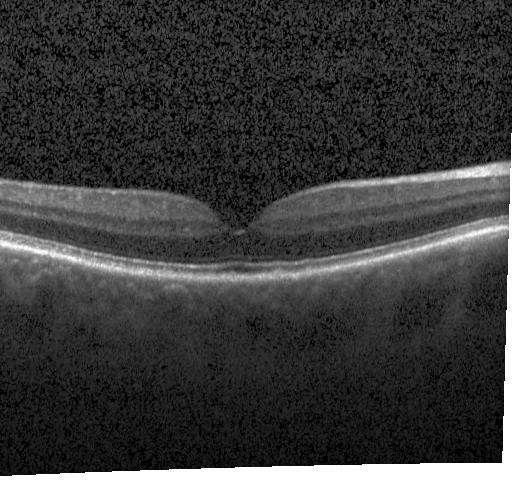 Diagnosis: neither choroidal neovascularization, diabetic macular edema, nor drusen.